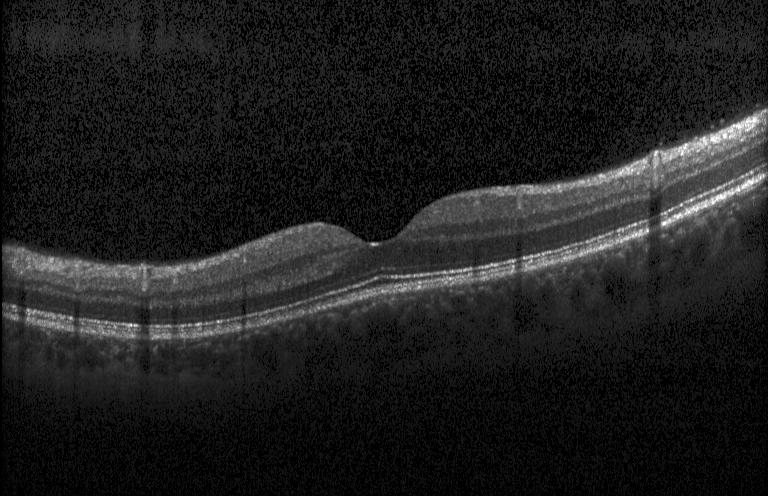 Horizontal scan through the fovea, Heidelberg Spectralis, optical coherence tomography scan, spectral-domain OCT
Impression: no CNV, no DME, and no drusen.